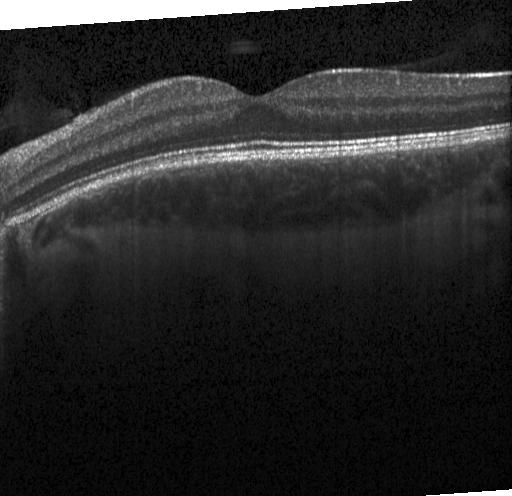

Instrument: Heidelberg Spectralis · optical coherence tomography scan — Impression: no CNV, no DME, and no drusen.